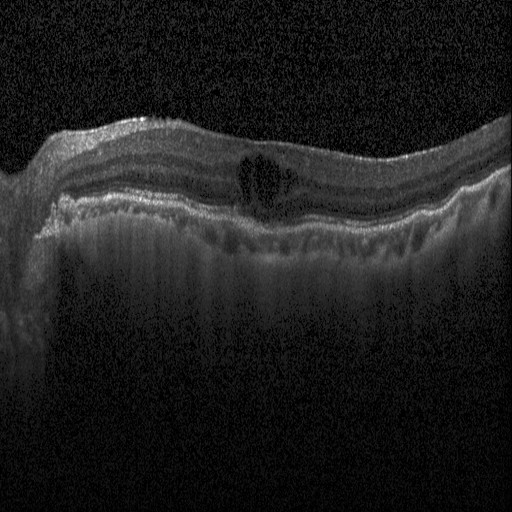 OCT line scan.
Macular OCT: diabetic macular edema.